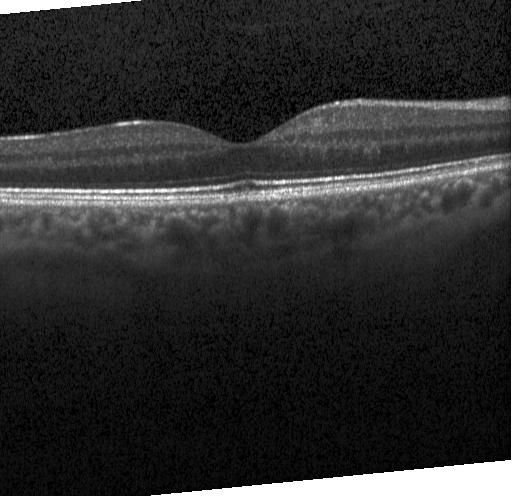
OCT line scan. Diagnosis: neither choroidal neovascularization, diabetic macular edema, nor drusen.